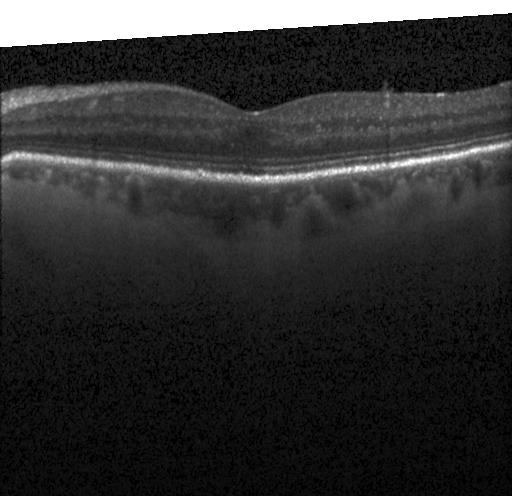 Impression: no CNV, no DME, and no drusen.